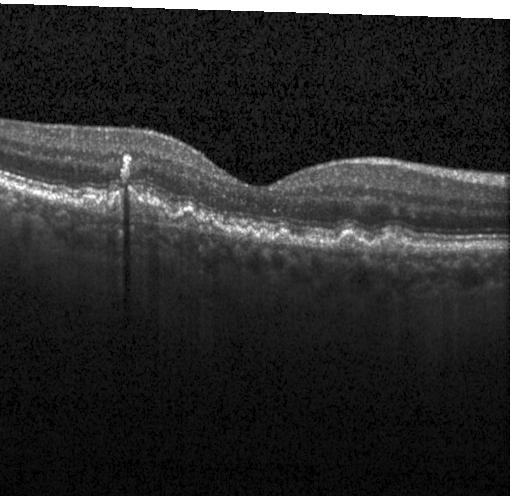

Retinal OCT B-scan. Spectral-domain OCT. Heidelberg Spectralis OCT system — The scan shows a choroidal neovascular membrane.